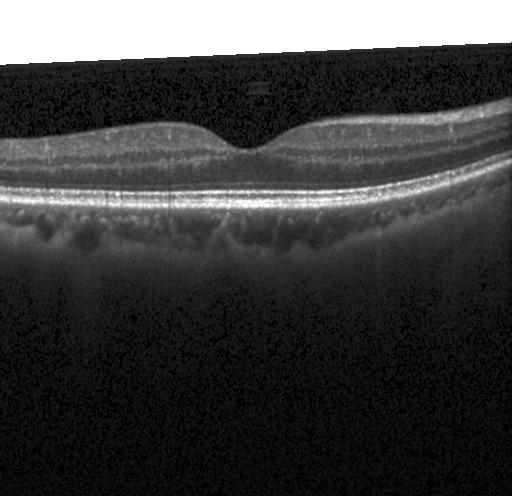 Heidelberg Spectralis OCT system · retinal OCT B-scan.
Dx: no choroidal neovascularization, no diabetic macular edema, and no drusen.